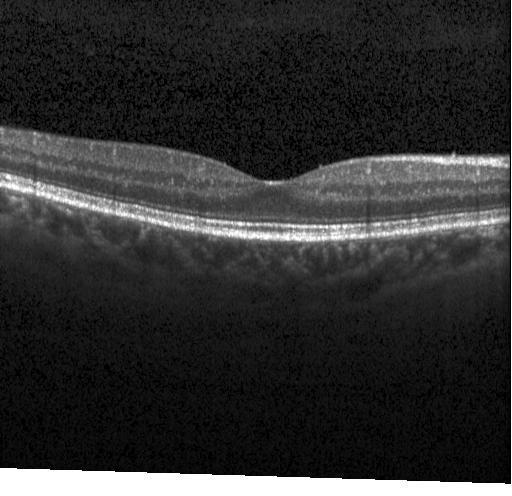 Retinal OCT cross-section — No choroidal neovascularization, no diabetic macular edema, and no drusen.